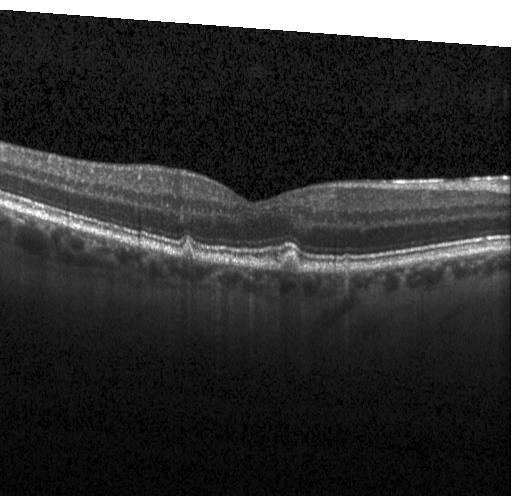 Retinal OCT cross-section. Through the macula
The scan shows sub-RPE drusenoid deposits.